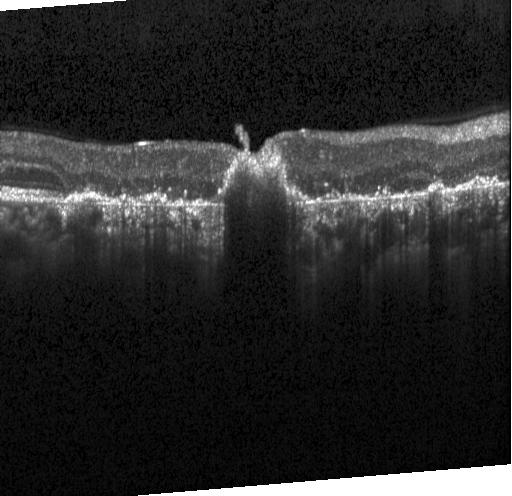

OCT scan showing a choroidal neovascular membrane.